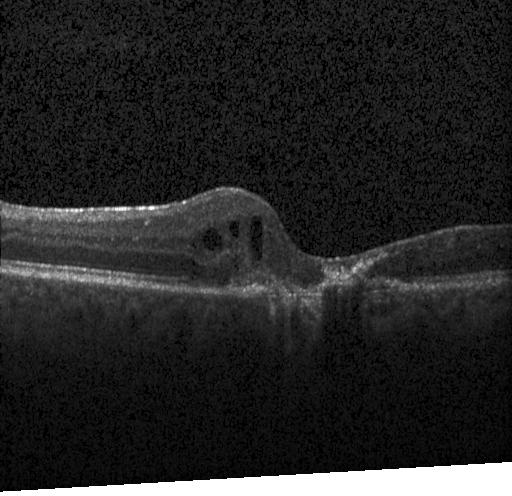

Choroidal neovascularization.